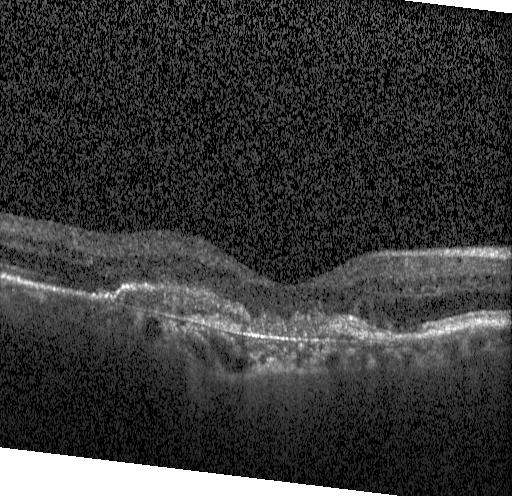
OCT line scan — This B-scan demonstrates CNV.